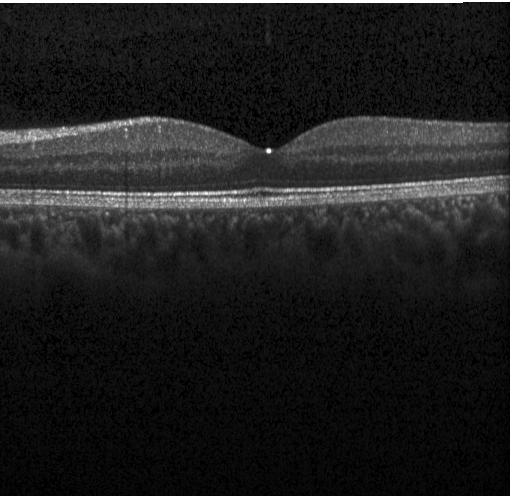 The scan shows no choroidal neovascularization, no diabetic macular edema, and no drusen.